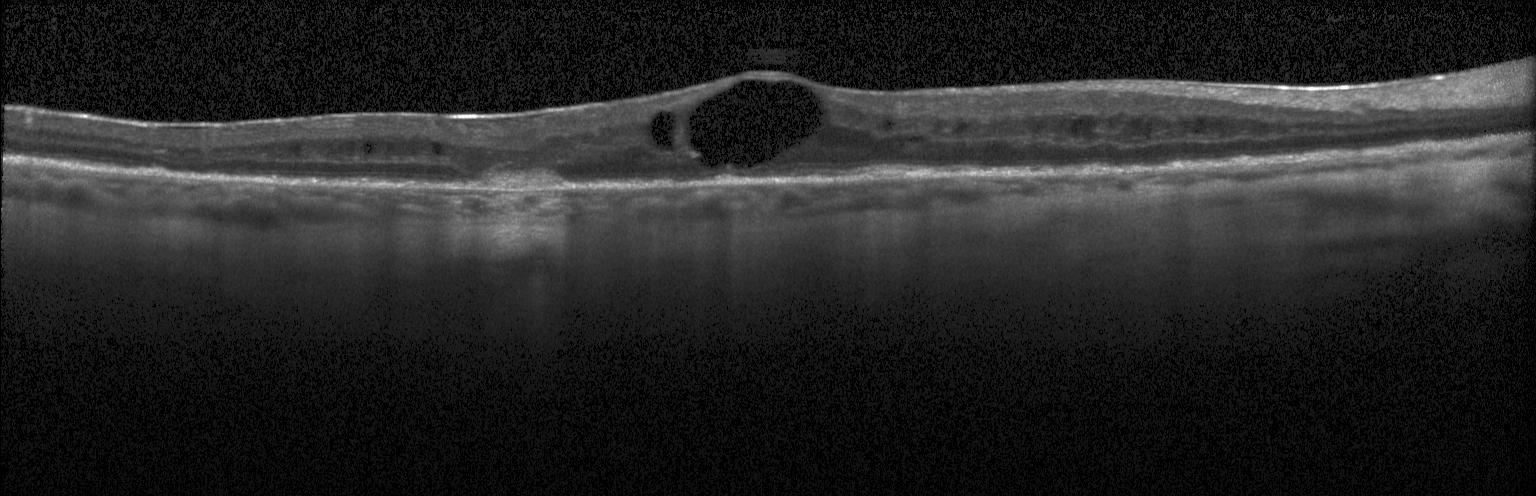
Optical coherence tomography scan · horizontal scan through the fovea. Diagnosis: a choroidal neovascular membrane.